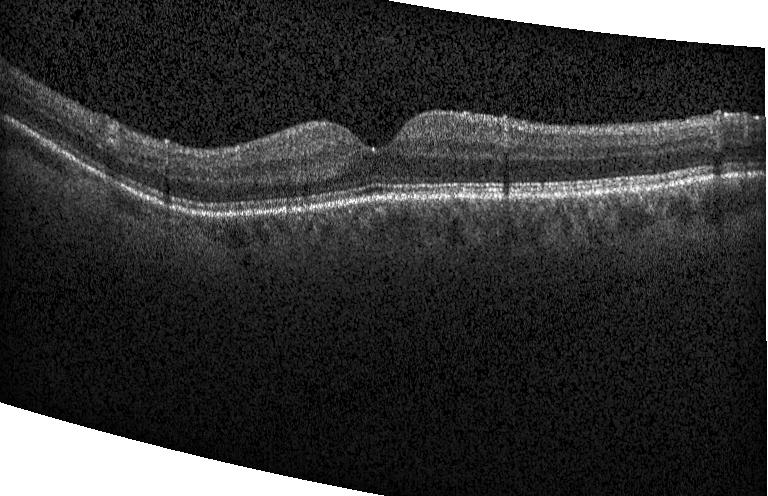

Instrument: Heidelberg Spectralis. Retinal OCT cross-section — Diagnosis: no choroidal neovascularization, no diabetic macular edema, and no drusen.